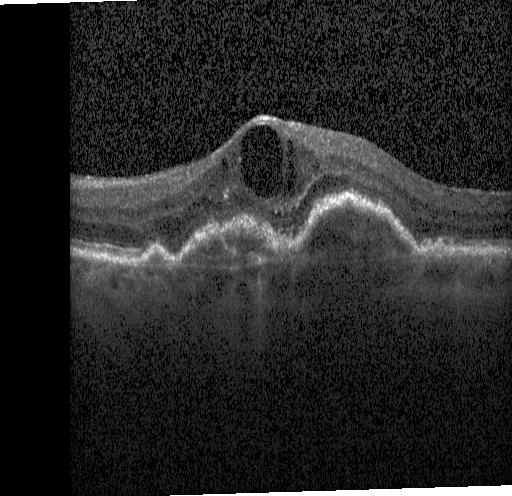 Macular OCT demonstrating a choroidal neovascular membrane.